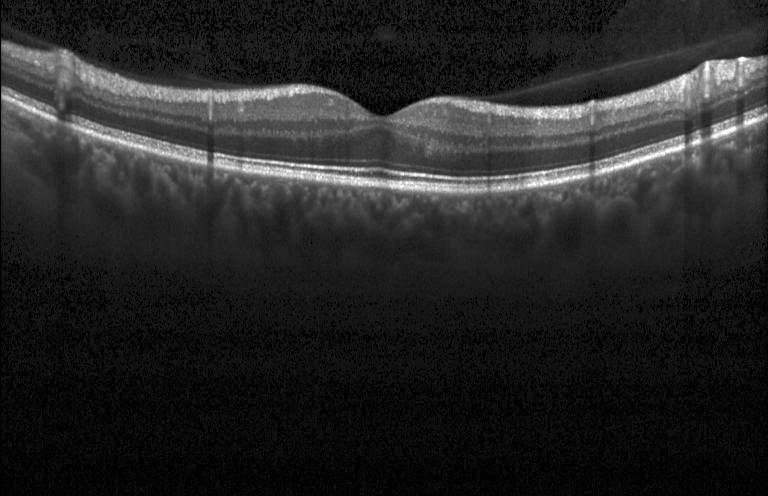
Macular scan. Retinal OCT cross-section. Spectral-domain OCT. Heidelberg Spectralis OCT system
Diagnosis: no CNV, DME, or drusen.